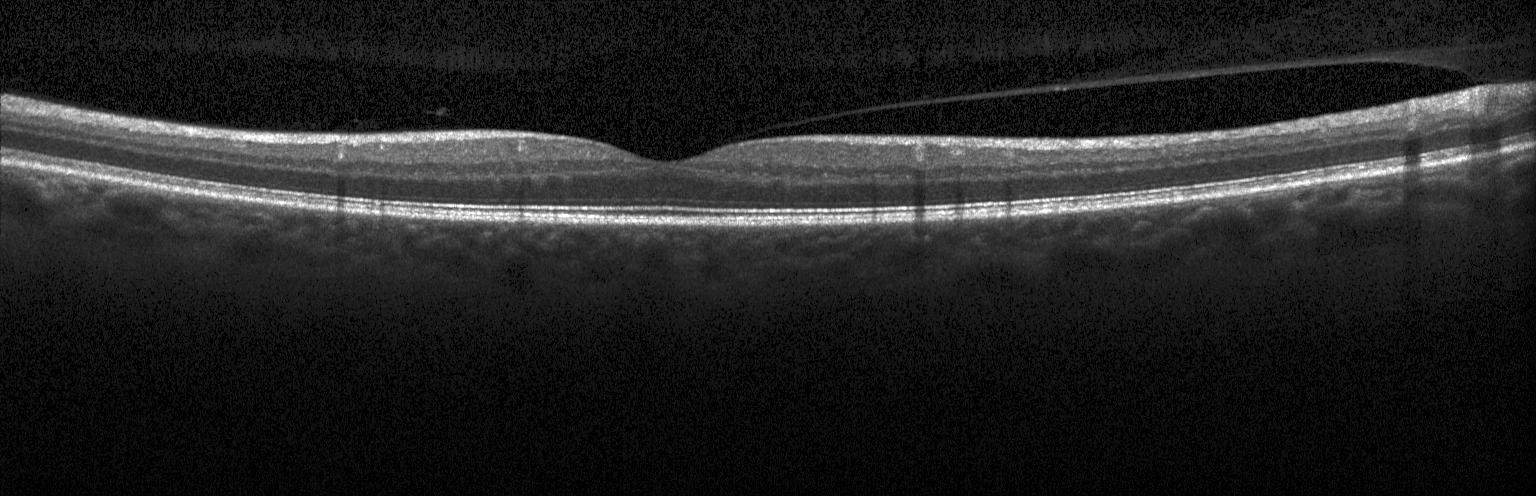

Impression: no choroidal neovascularization, diabetic macular edema, or drusen.